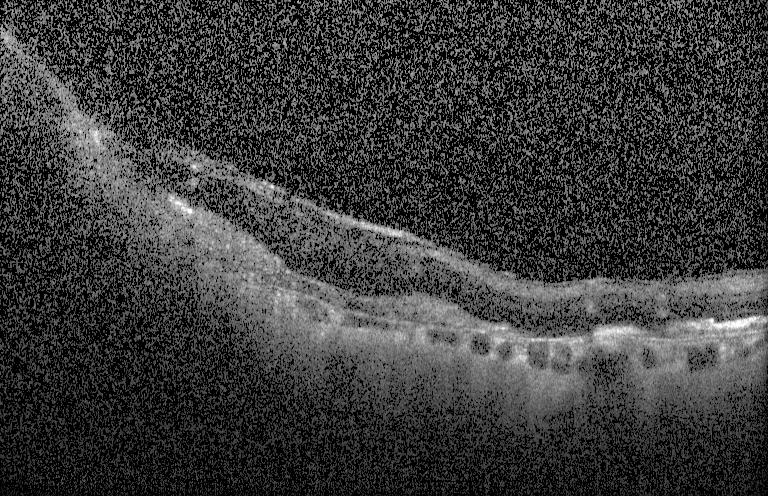
Heidelberg Spectralis, OCT B-scan.
Assessment: a choroidal neovascular membrane.